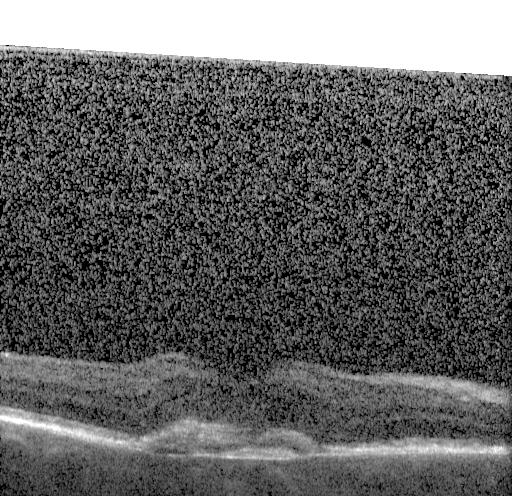
Retinal OCT cross-section, spectral-domain optical coherence tomography. Impression: a choroidal neovascular membrane.